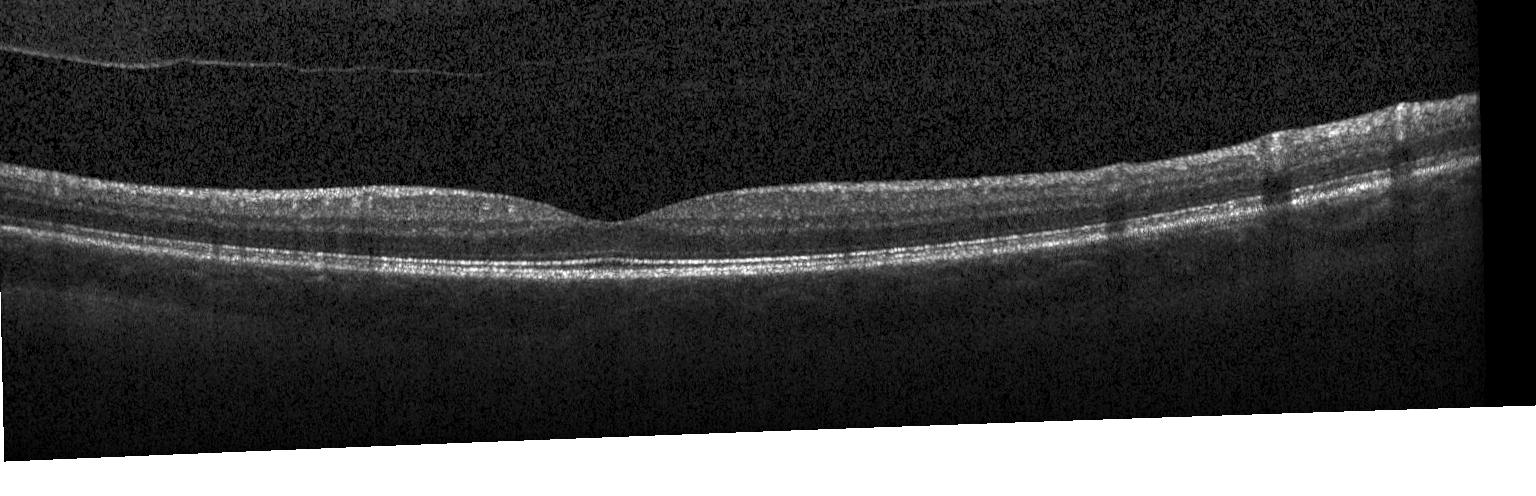 Optical coherence tomography scan; macular scan; spectral-domain optical coherence tomography; acquired on a Heidelberg Spectralis.
Macular OCT: no evidence of CNV, DME, or drusen.